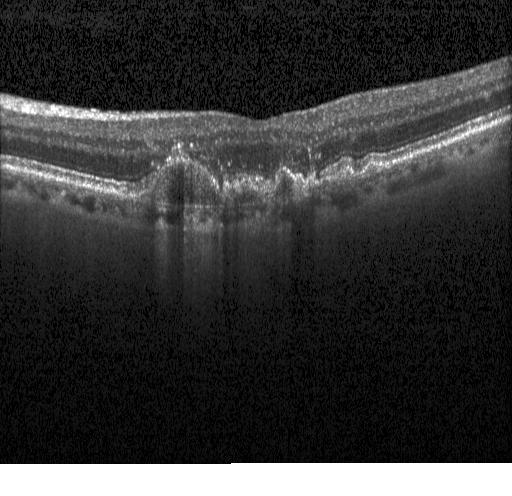 OCT B-scan. Centered on the fovea. Macular OCT: choroidal neovascularization (CNV).